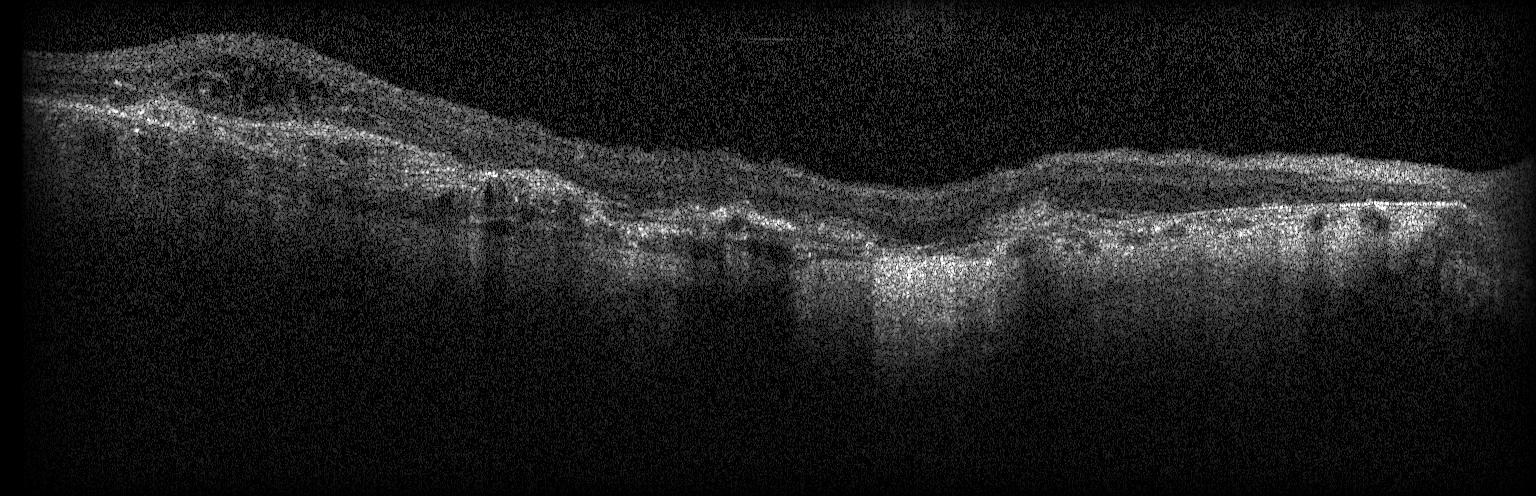
Retinal OCT B-scan. Instrument: Heidelberg Spectralis. Macular scan.
Impression: a choroidal neovascular membrane.